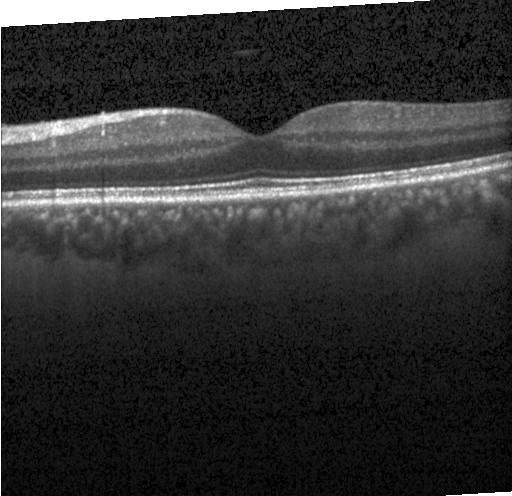

Optical coherence tomography scan · acquired on a Heidelberg Spectralis — Diagnosis: no CNV, no DME, and no drusen.